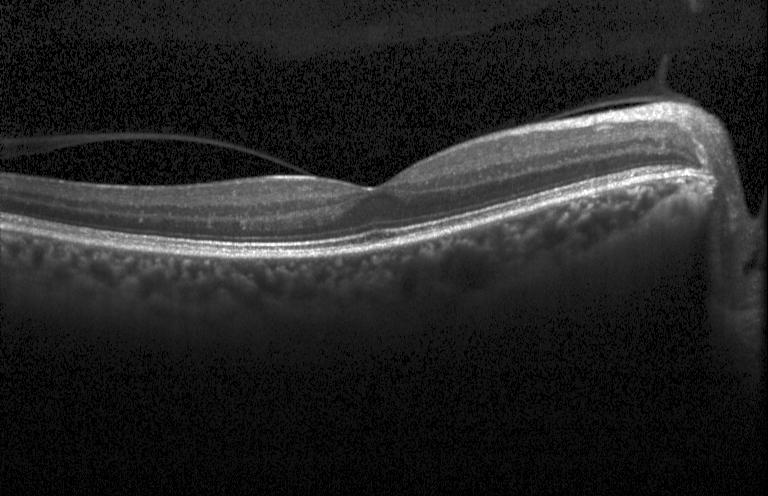
Impression: neither choroidal neovascularization, diabetic macular edema, nor drusen.